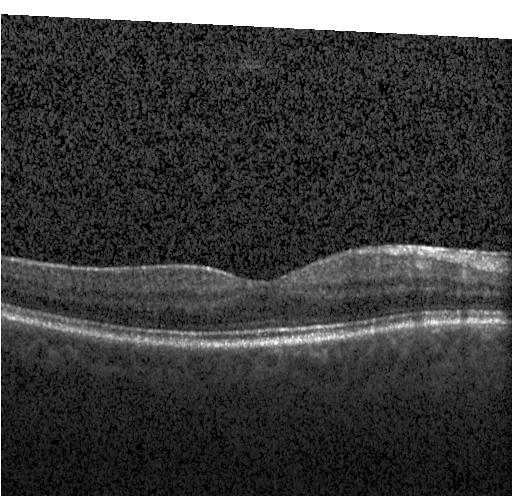

Finding: neither choroidal neovascularization, diabetic macular edema, nor drusen.